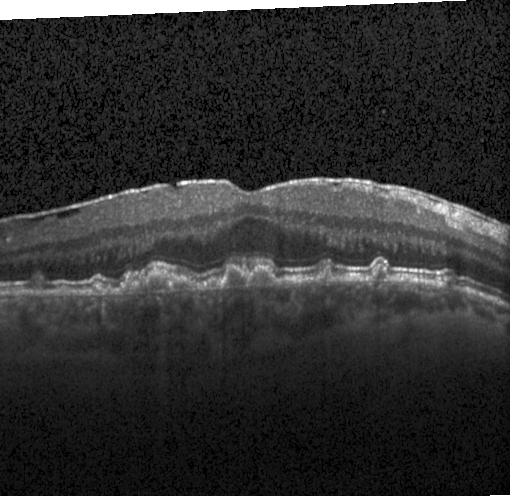

Spectral-domain optical coherence tomography. OCT line scan — CNV.